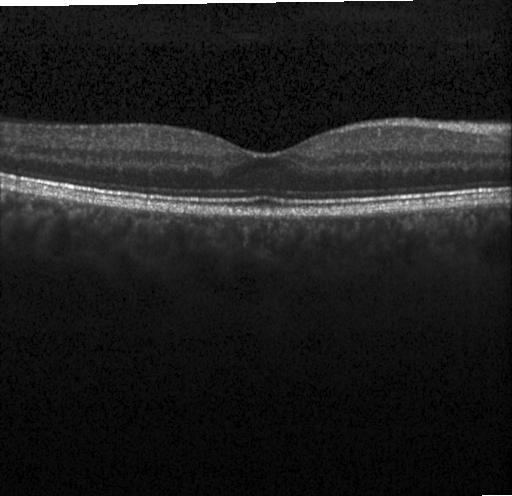 Spectral-domain optical coherence tomography · OCT B-scan.
Dx: no CNV, no DME, and no drusen.